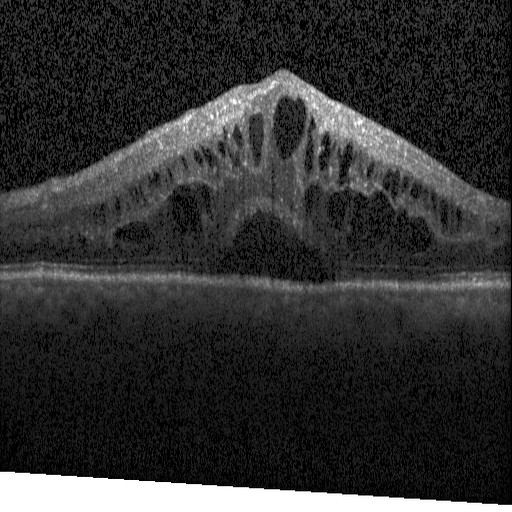 OCT scan showing diabetic macular edema (DME).